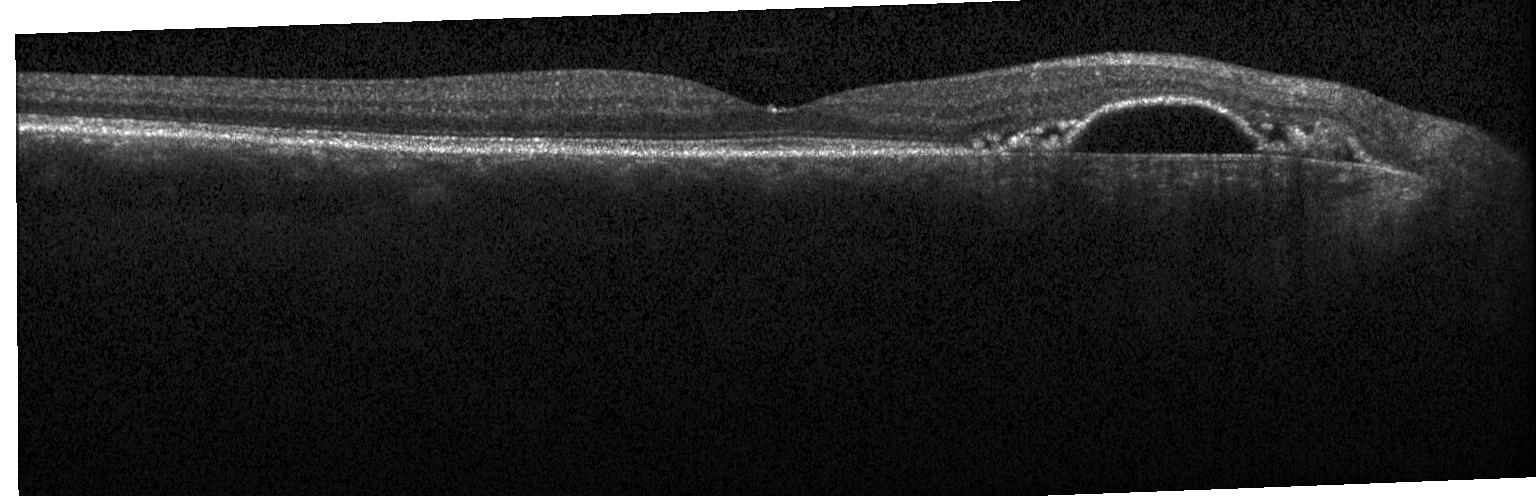

OCT B-scan, spectral-domain OCT
This B-scan demonstrates choroidal neovascularization.